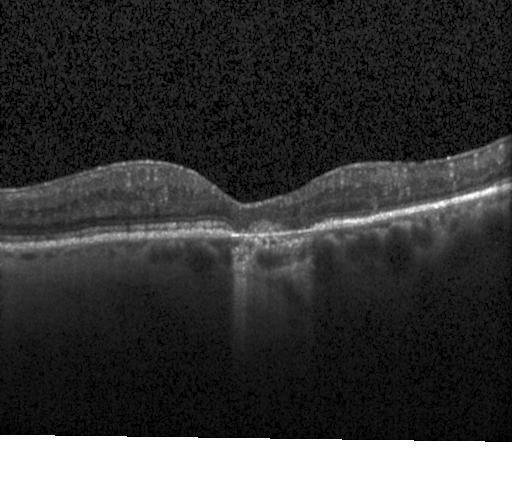
OCT B-scan. SD-OCT. Instrument: Heidelberg Spectralis. Macular scan. Diagnosis: a choroidal neovascular membrane.